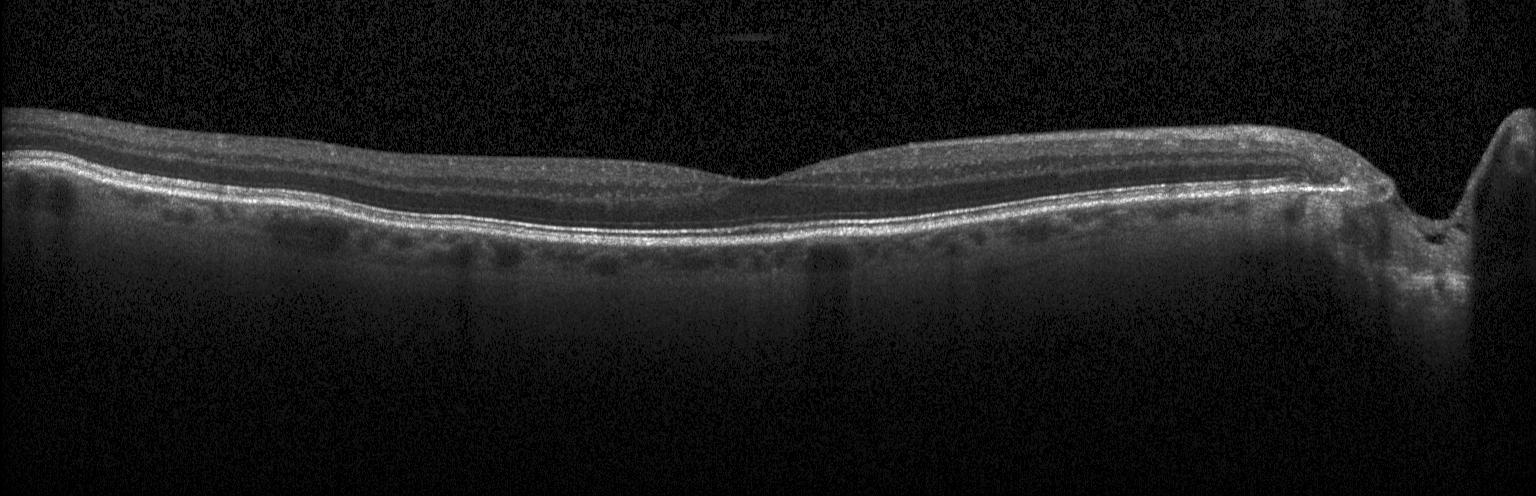
Retinal OCT cross-section showing no evidence of choroidal neovascularization, diabetic macular edema, or drusen.